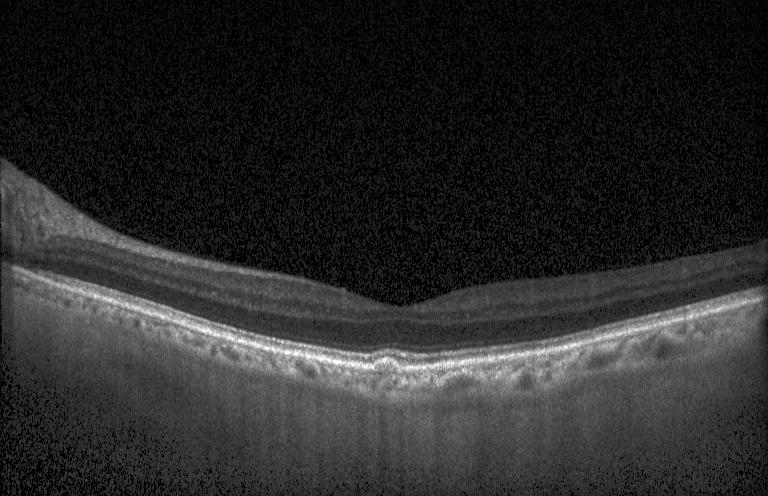 Dx: multiple drusen.